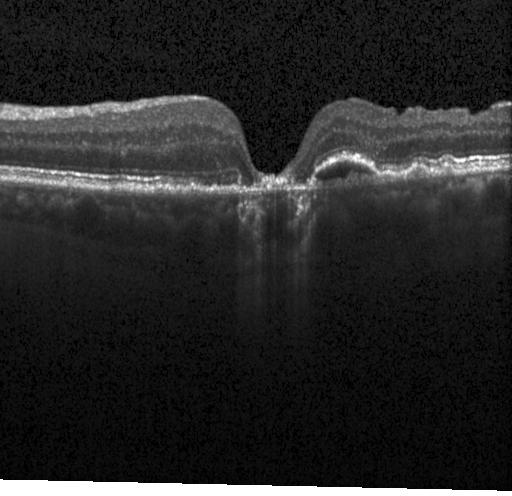
Optical coherence tomography B-scan. Spectral-domain OCT
A choroidal neovascular membrane.